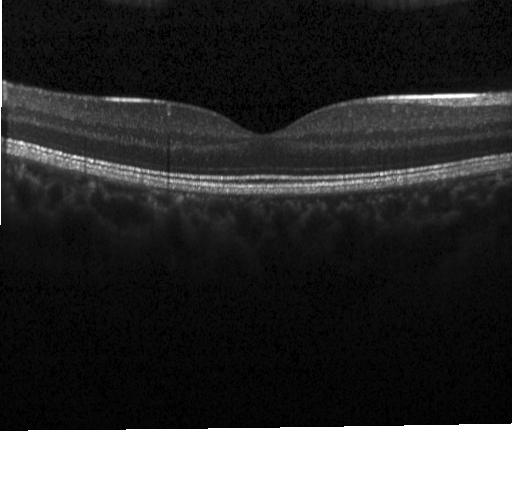
Retinal OCT cross-section. Spectral-domain optical coherence tomography.
Dx: no choroidal neovascularization, no diabetic macular edema, and no drusen.